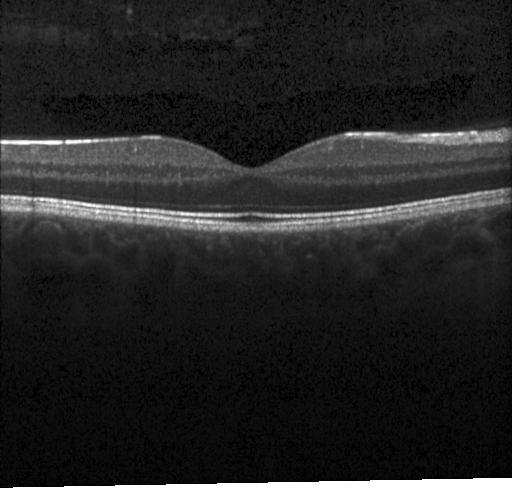 Finding: neither CNV, DME, nor drusen.